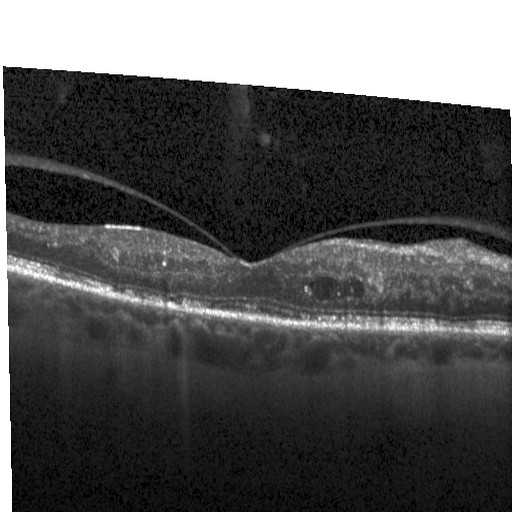
Impression: diabetic macular edema (DME).